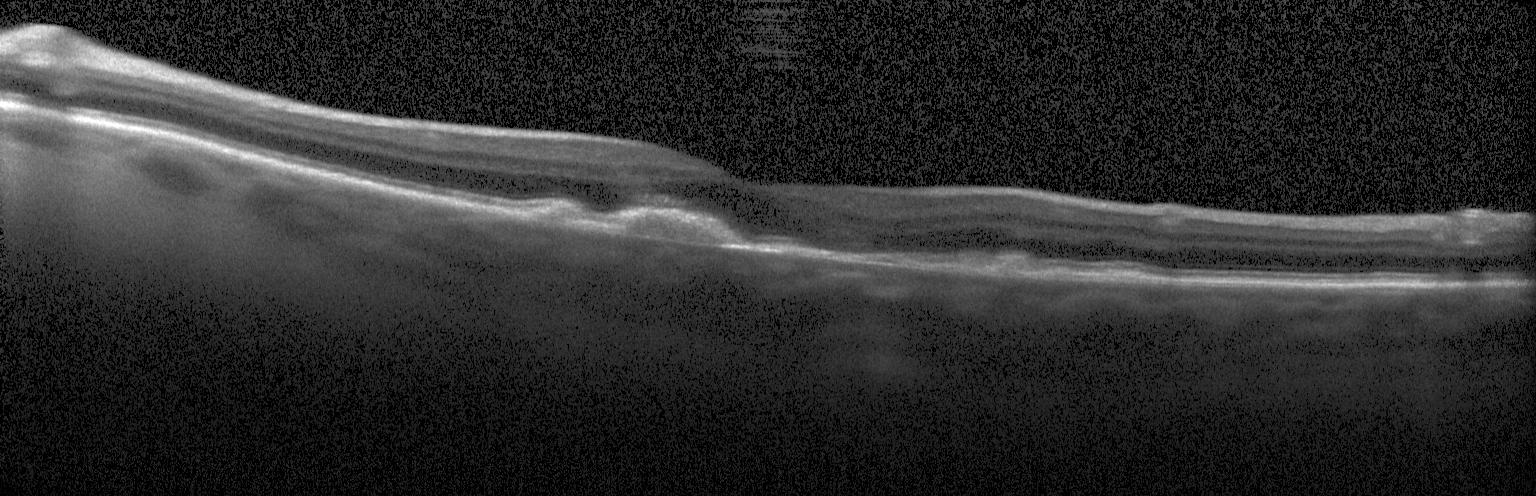
Heidelberg Spectralis; retinal OCT cross-section — OCT finding: a choroidal neovascular membrane.